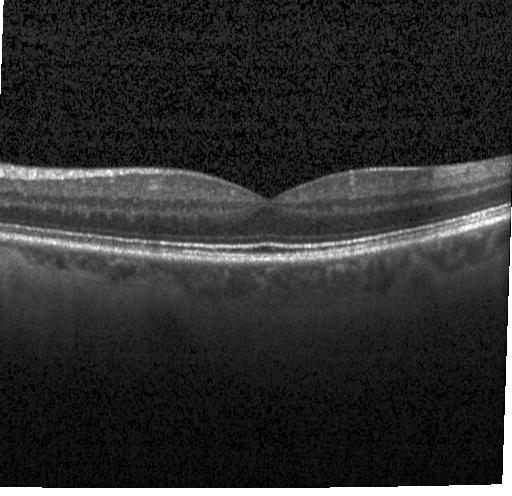
Diagnosis: no choroidal neovascularization, diabetic macular edema, or drusen.